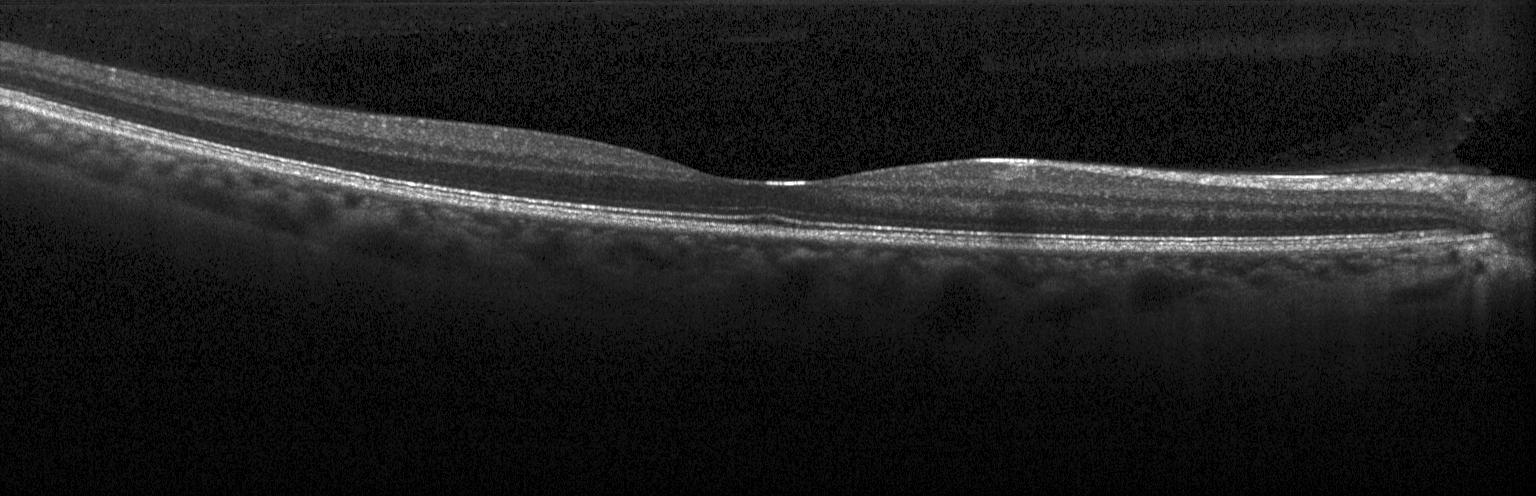 Optical coherence tomography scan · acquired on a Heidelberg Spectralis. This B-scan demonstrates no CNV, DME, or drusen.